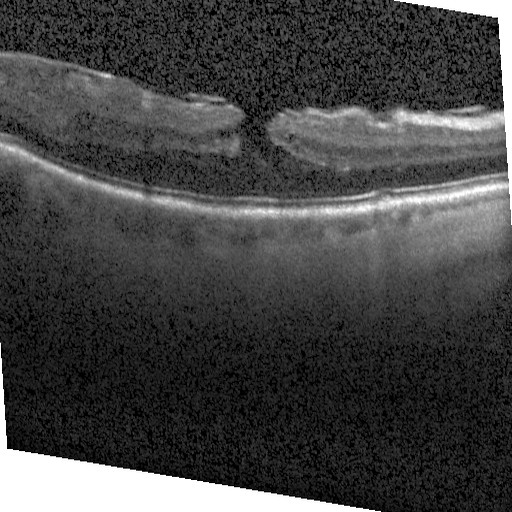

OCT scan showing DME.